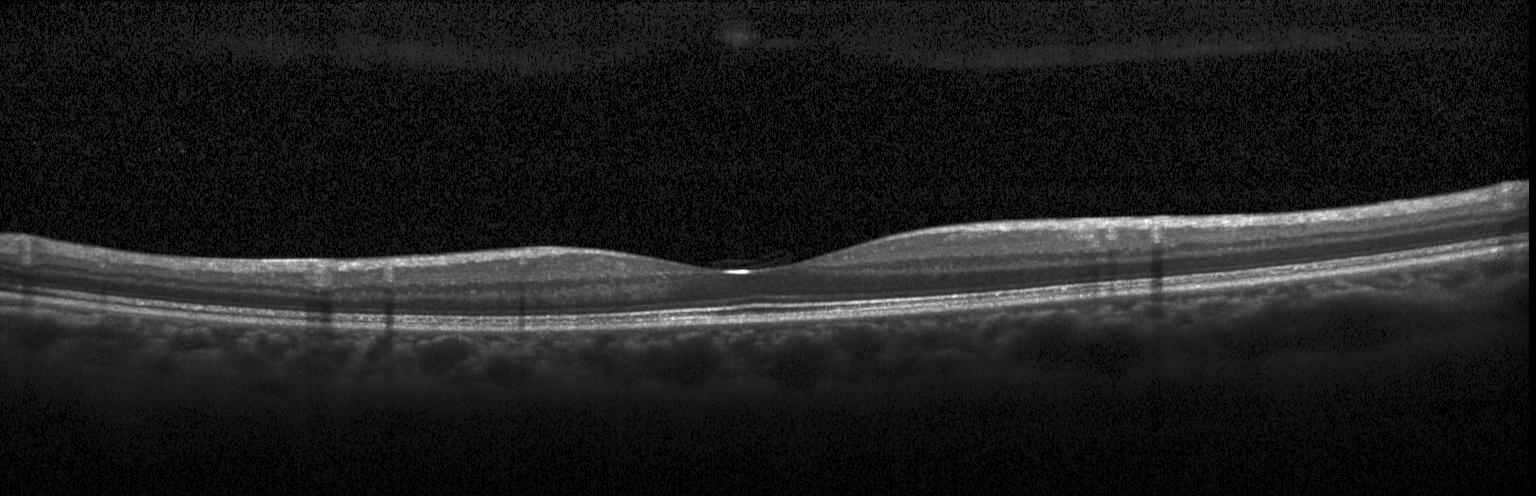
Assessment: neither choroidal neovascularization, diabetic macular edema, nor drusen.